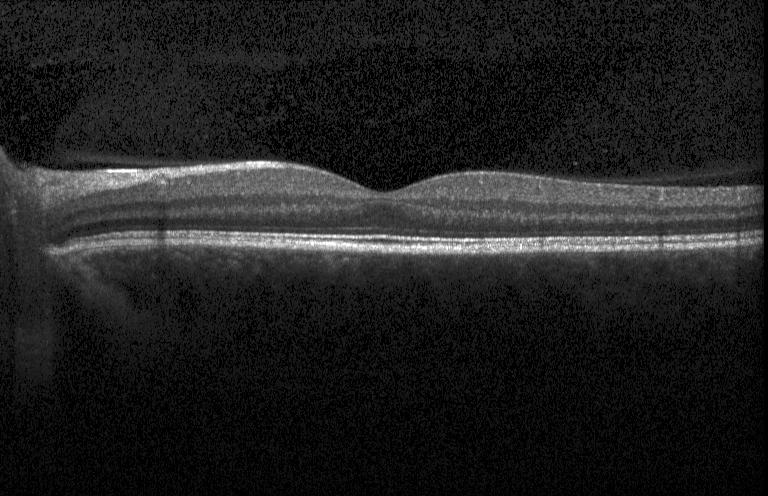

Optical coherence tomography scan, spectral-domain optical coherence tomography — Impression: no CNV, DME, or drusen.